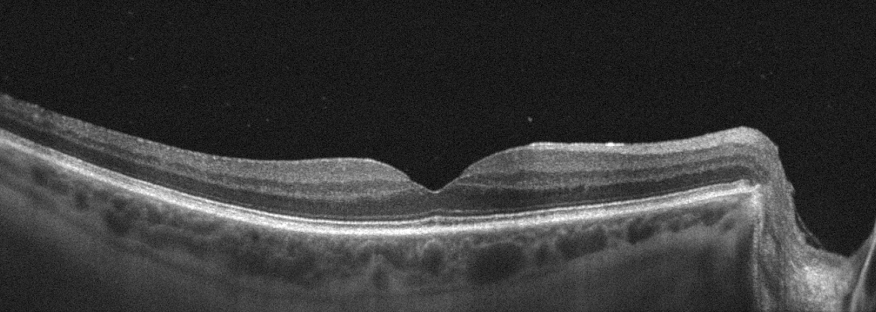
Diagnosis: age-related macular degeneration (AMD).